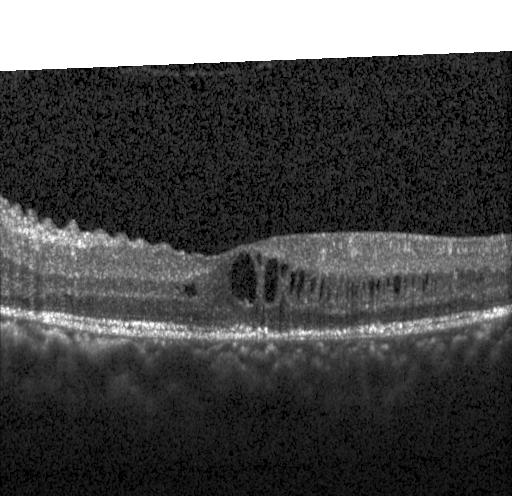

Finding: DME.